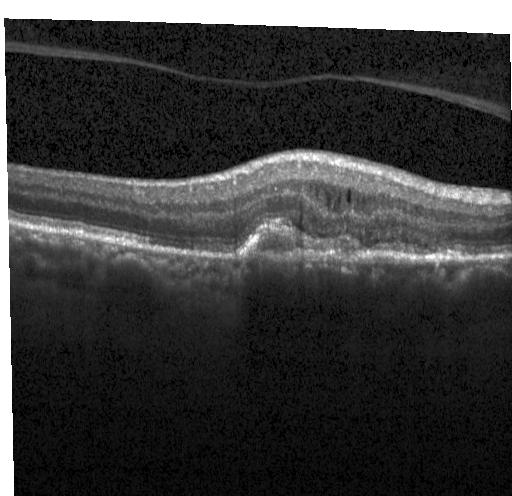 Spectral-domain optical coherence tomography · instrument: Heidelberg Spectralis · OCT line scan · horizontal scan through the fovea.
Finding: choroidal neovascularization (CNV).